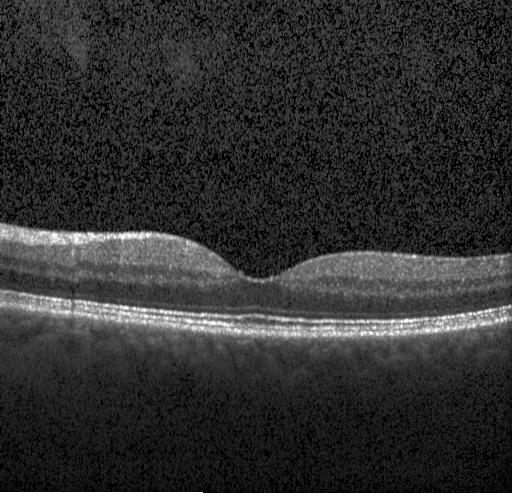
OCT B-scan showing no evidence of choroidal neovascularization, diabetic macular edema, or drusen.